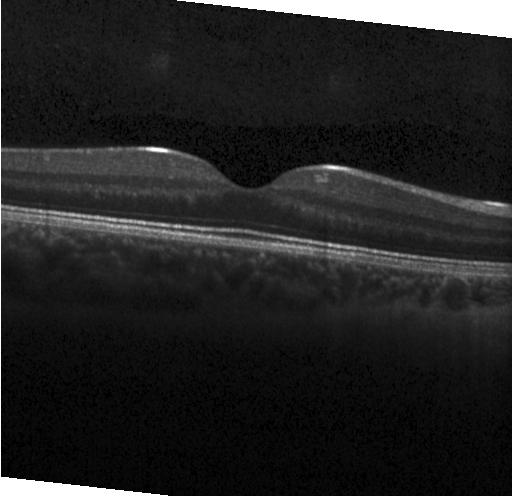
Spectral-domain OCT. Heidelberg Spectralis. Retinal OCT B-scan. Macular scan
Assessment: no evidence of choroidal neovascularization, diabetic macular edema, or drusen.